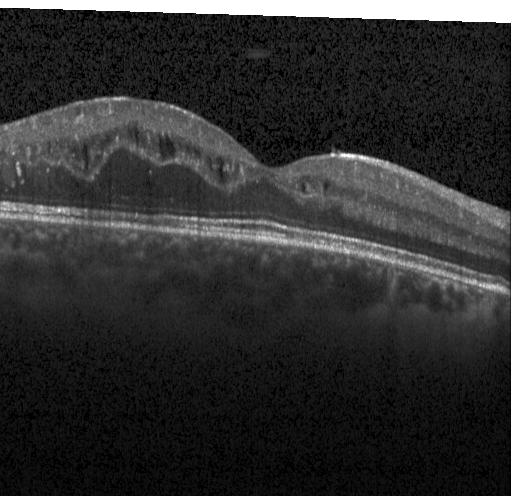

Fovea-centered; Heidelberg Spectralis; retinal OCT cross-section; spectral-domain OCT — Finding: diabetic macular edema (DME).